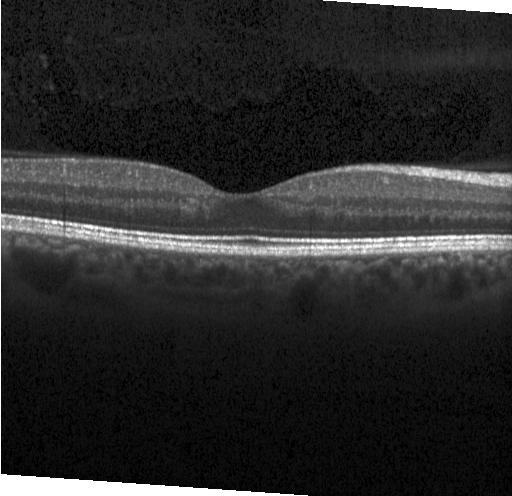
No evidence of choroidal neovascularization, diabetic macular edema, or drusen.